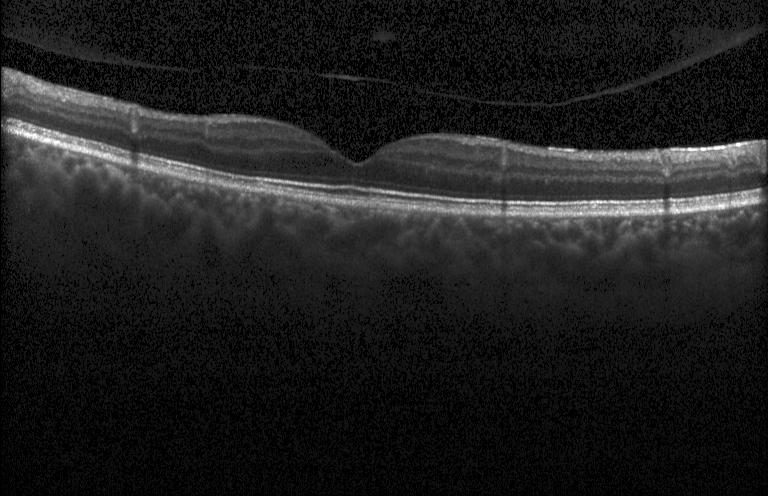

Fovea-centered · Heidelberg Spectralis OCT system · optical coherence tomography scan
Neither CNV, DME, nor drusen.